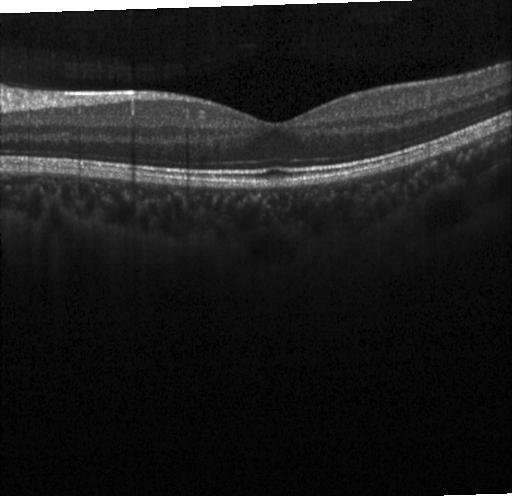

Optical coherence tomography B-scan.
Assessment: no evidence of CNV, DME, or drusen.